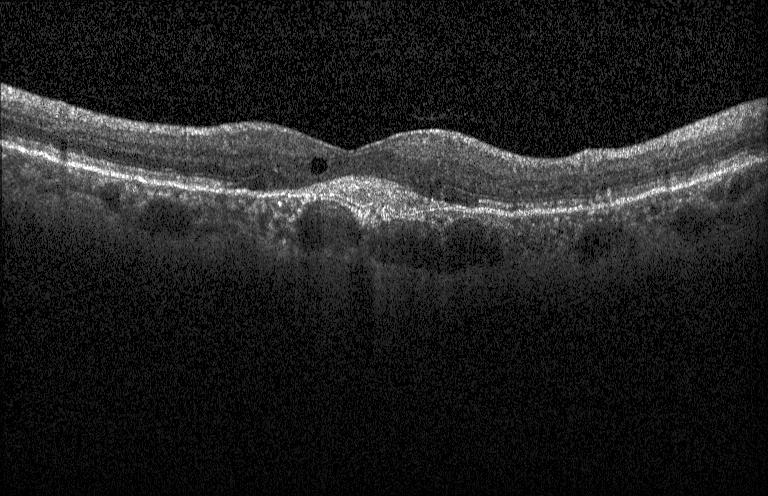
Impression: a choroidal neovascular membrane.